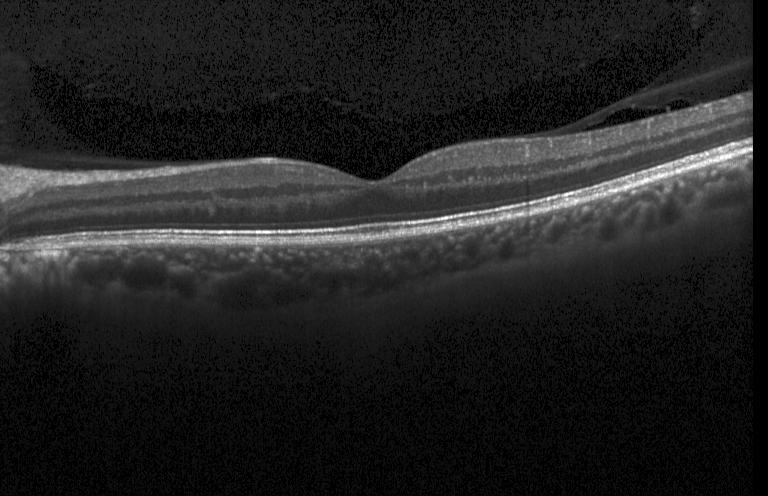
Macular OCT demonstrating no choroidal neovascularization, no diabetic macular edema, and no drusen.